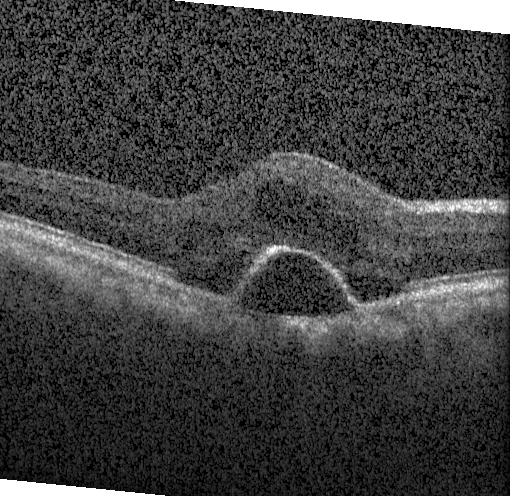

SD-OCT. Retinal OCT cross-section. Horizontal scan through the fovea — Finding: choroidal neovascularization.